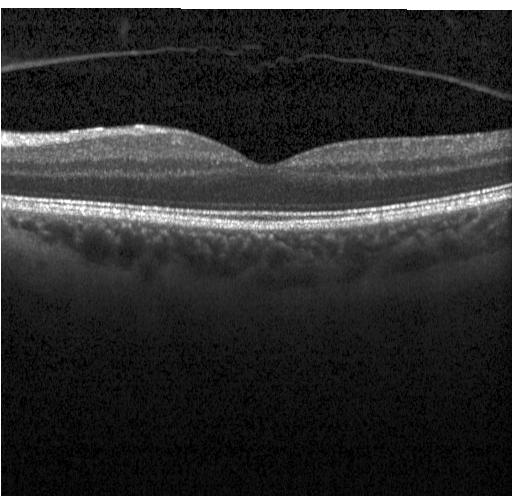 Impression: neither choroidal neovascularization, diabetic macular edema, nor drusen.